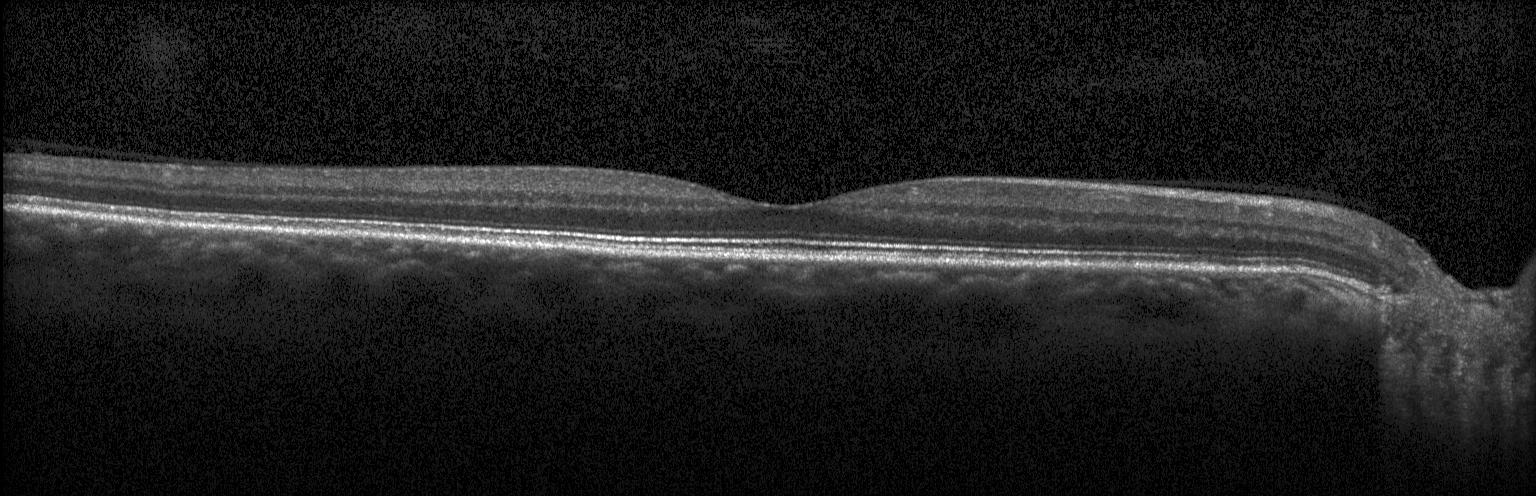 Dx: no choroidal neovascularization, diabetic macular edema, or drusen.